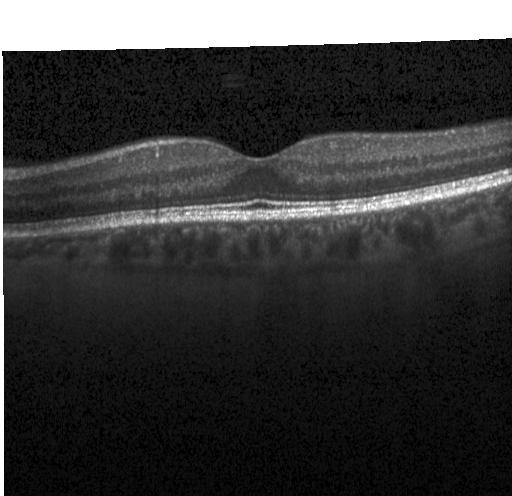 Retinal OCT cross-section; Heidelberg Spectralis — This B-scan demonstrates no evidence of choroidal neovascularization, diabetic macular edema, or drusen.